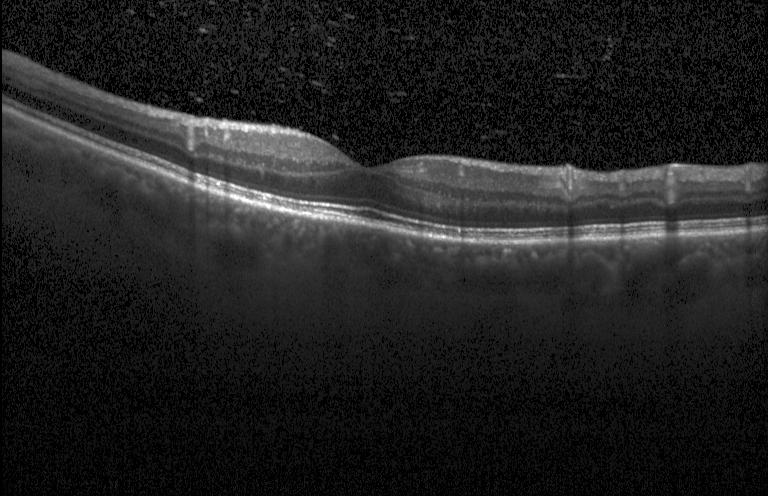
Optical coherence tomography B-scan — Finding: no evidence of choroidal neovascularization, diabetic macular edema, or drusen.